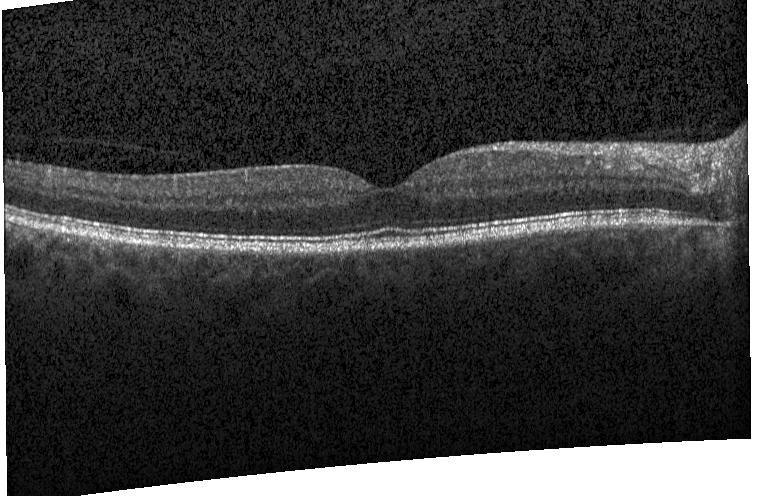

Finding: no CNV, DME, or drusen.